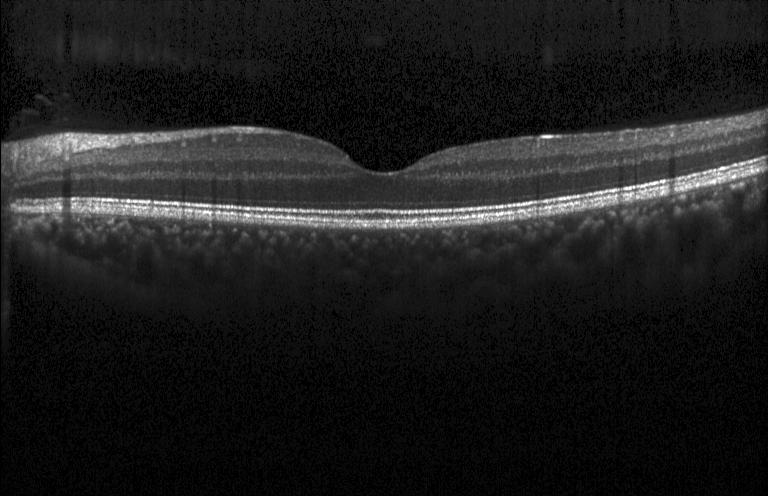 Dx: no choroidal neovascularization, no diabetic macular edema, and no drusen.